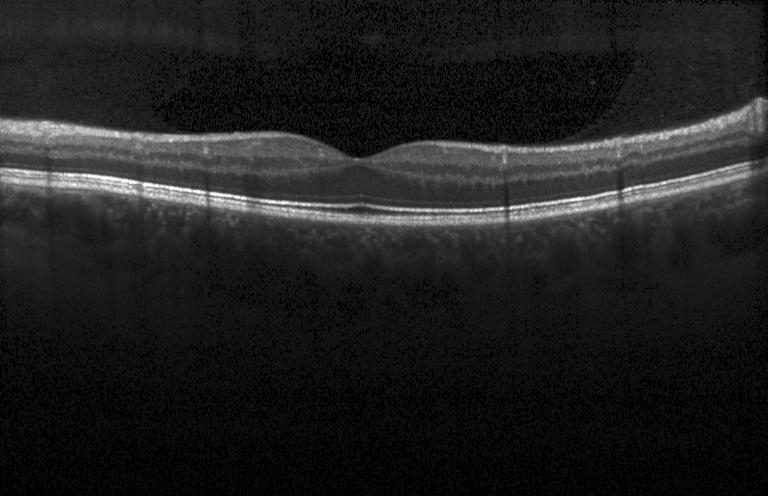

Retinal OCT B-scan · spectral-domain optical coherence tomography · through the macula · instrument: Heidelberg Spectralis.
Diagnosis: no choroidal neovascularization, diabetic macular edema, or drusen.